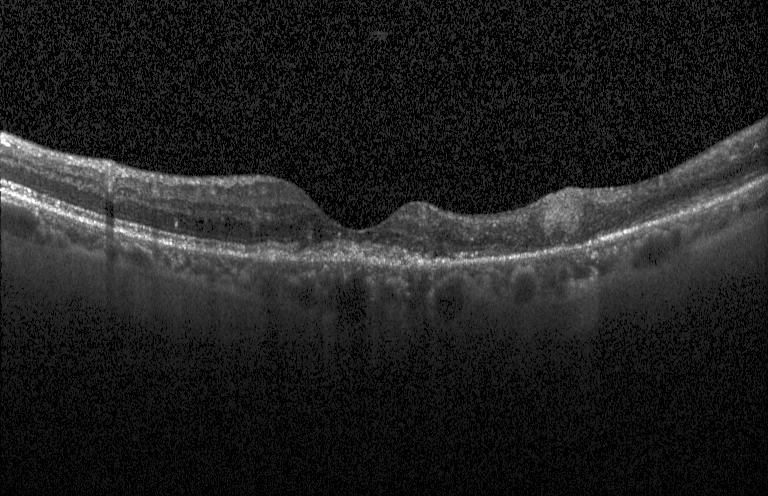
Retinal OCT cross-section — Impression: a choroidal neovascular membrane.